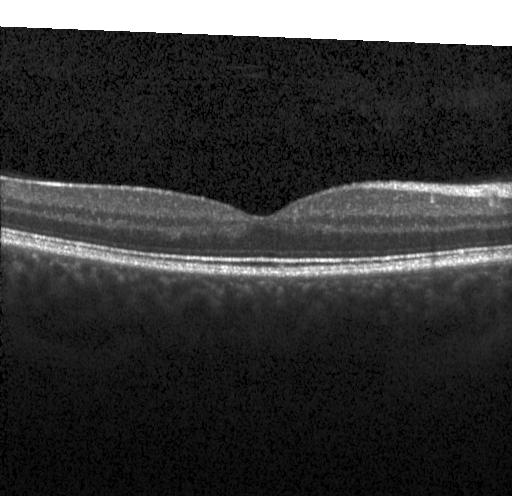

SD-OCT · optical coherence tomography B-scan · through the macula. Diagnosis: no evidence of choroidal neovascularization, diabetic macular edema, or drusen.